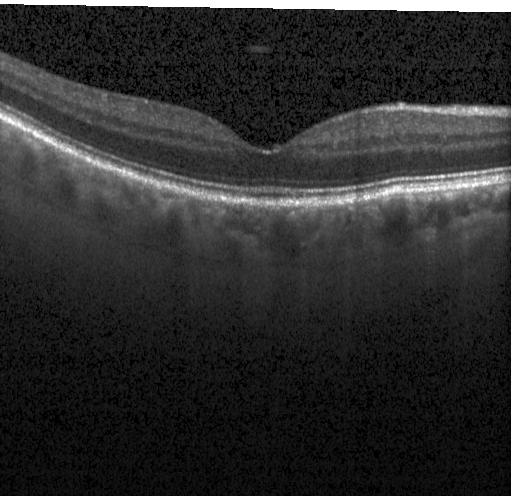

Macular OCT demonstrating no evidence of choroidal neovascularization, diabetic macular edema, or drusen.